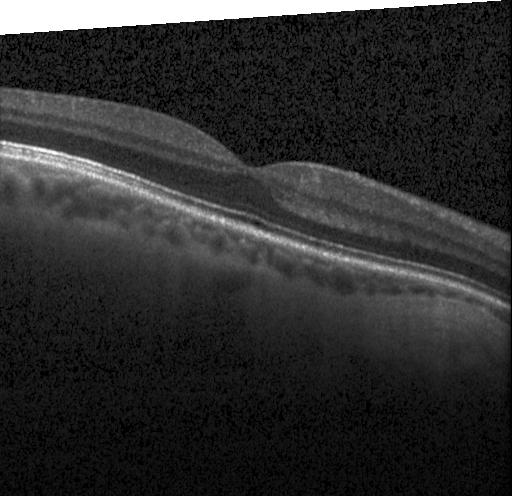
Macular OCT demonstrating neither choroidal neovascularization, diabetic macular edema, nor drusen.